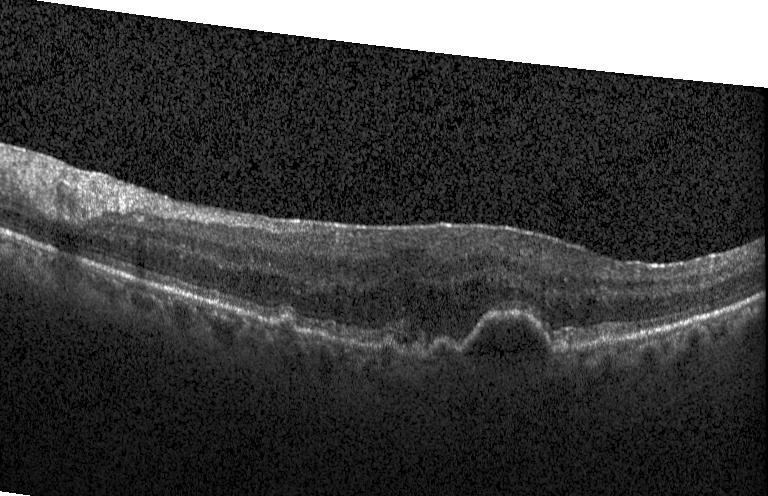
This B-scan demonstrates a choroidal neovascular membrane.